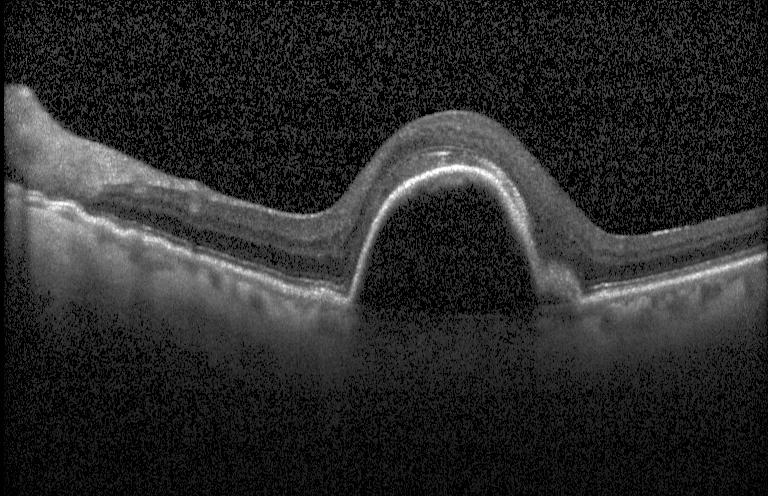
Retinal OCT B-scan
Assessment: a choroidal neovascular membrane.